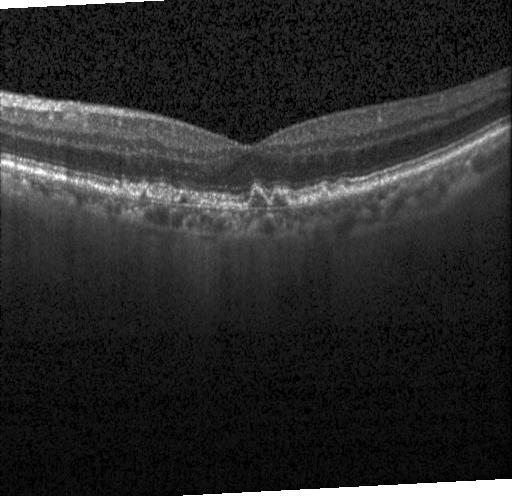 Centered on the fovea; spectral-domain optical coherence tomography; acquired on a Heidelberg Spectralis; OCT line scan.
Finding: drusen.